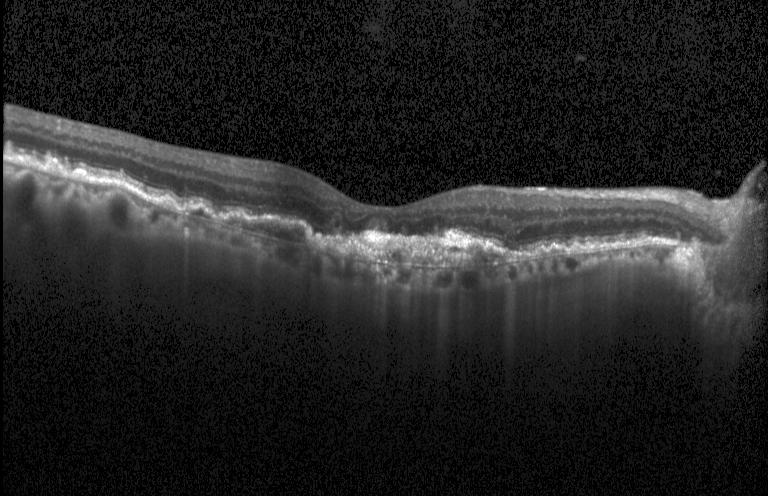

Optical coherence tomography scan — Assessment: a choroidal neovascular membrane.